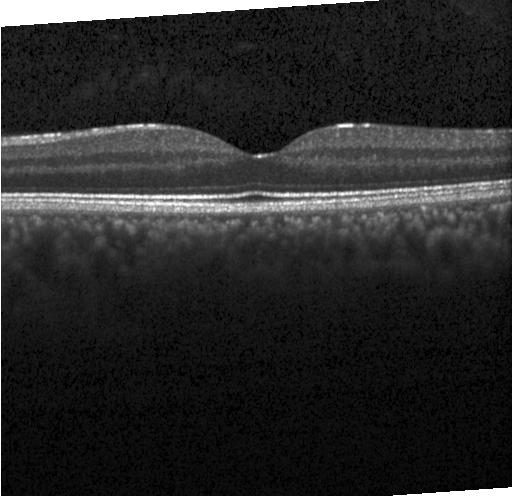 The scan shows no choroidal neovascularization, diabetic macular edema, or drusen.